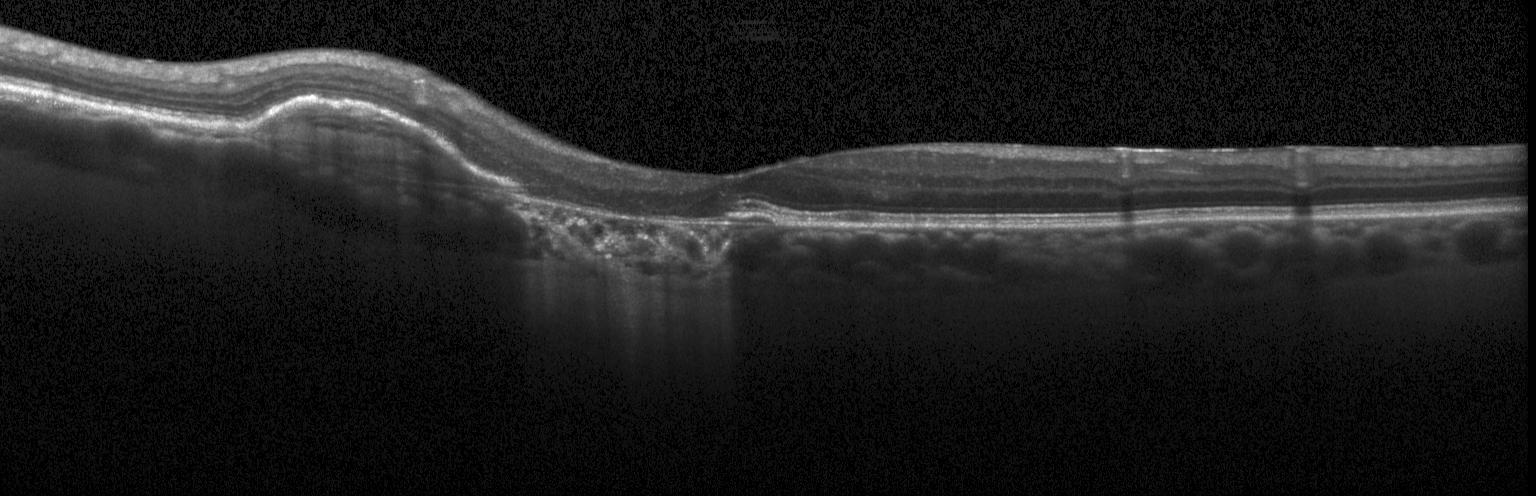
Spectral-domain optical coherence tomography; acquired on a Heidelberg Spectralis; retinal OCT cross-section; fovea-centered
Dx: choroidal neovascularization.